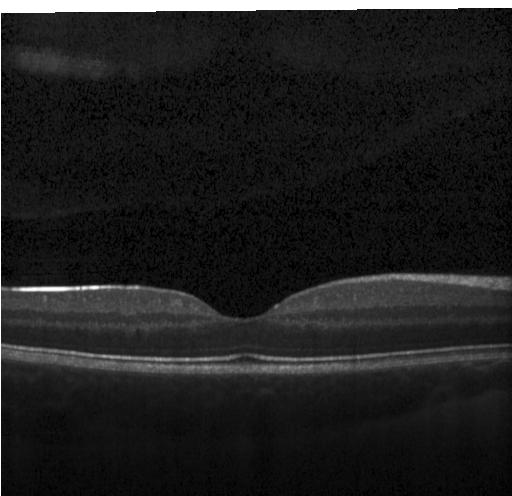

Retinal OCT cross-section showing no evidence of CNV, DME, or drusen.